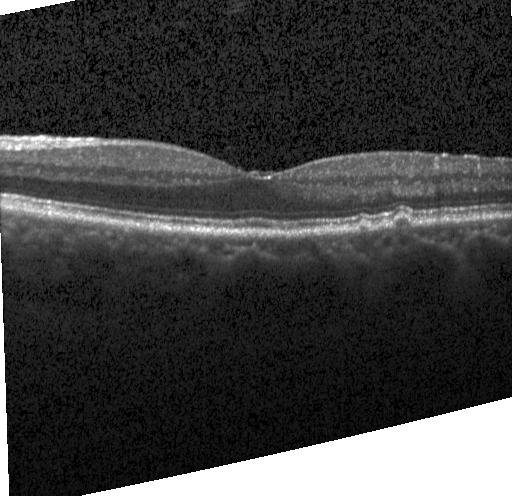 Finding: sub-RPE drusenoid deposits.